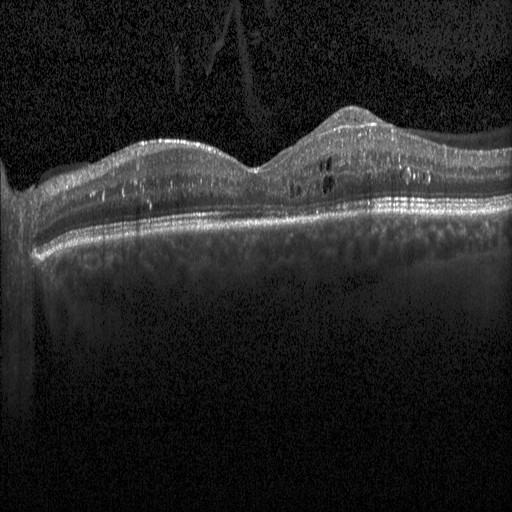
Heidelberg Spectralis OCT system; fovea-centered; retinal OCT cross-section; spectral-domain optical coherence tomography
Assessment: diabetic macular edema (DME).